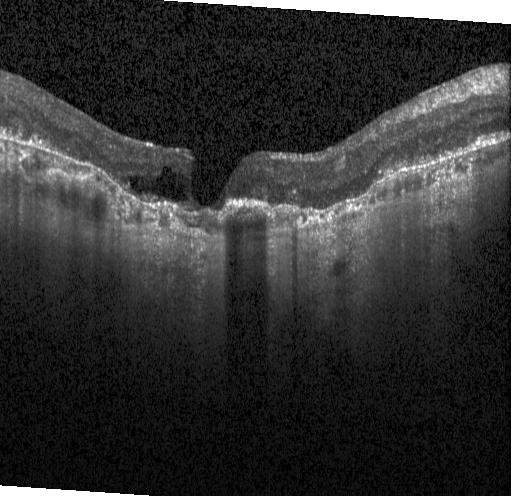
OCT line scan.
Macular OCT: a choroidal neovascular membrane.